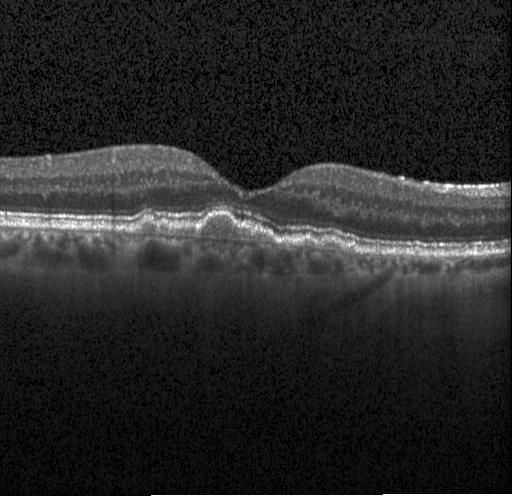 Spectral-domain OCT. Optical coherence tomography scan. Centered on the fovea. Heidelberg Spectralis
Assessment: drusen.